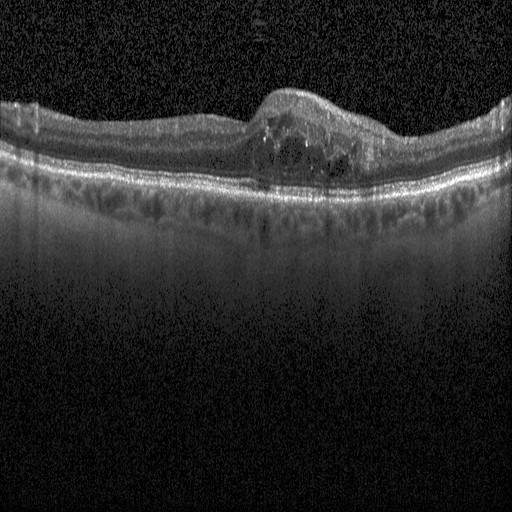 Finding: diabetic macular edema (DME).